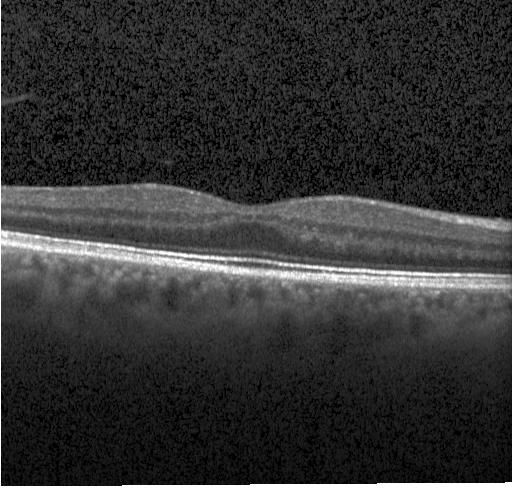 Acquired on a Heidelberg Spectralis · spectral-domain optical coherence tomography · optical coherence tomography B-scan.
Dx: no choroidal neovascularization, diabetic macular edema, or drusen.